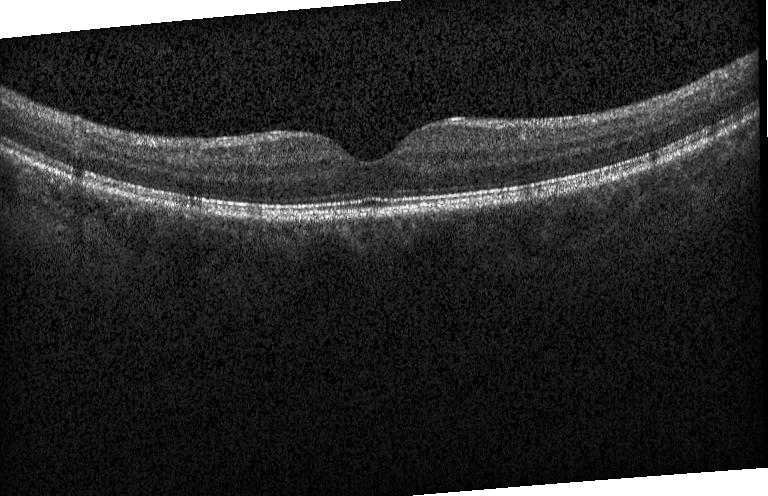 OCT line scan, fovea-centered.
Impression: no choroidal neovascularization, no diabetic macular edema, and no drusen.